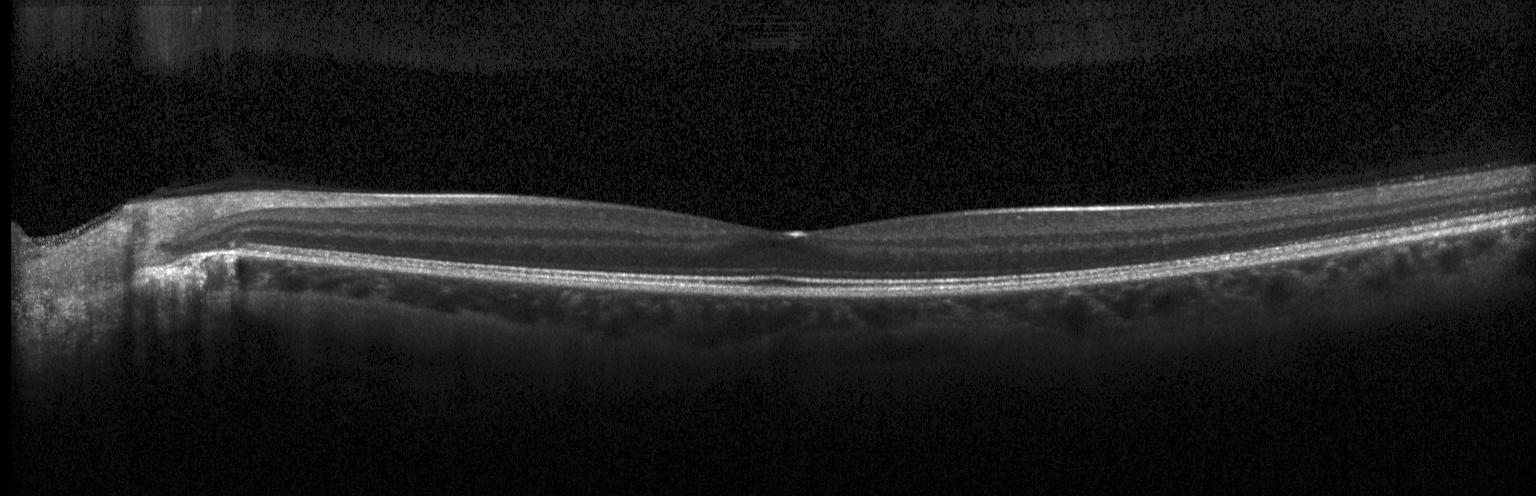

Finding: no CNV, DME, or drusen.